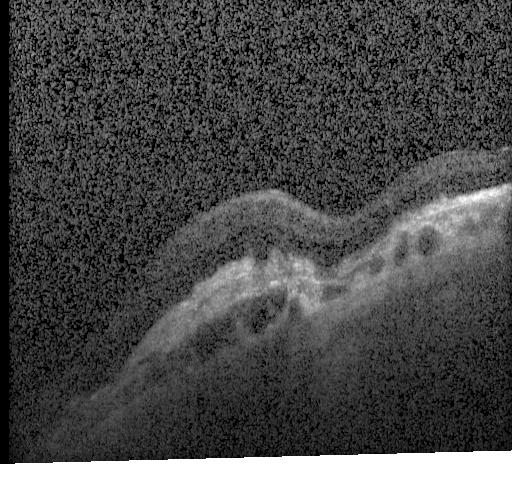
Macular scan; Heidelberg Spectralis; OCT line scan.
This B-scan demonstrates choroidal neovascularization (CNV).